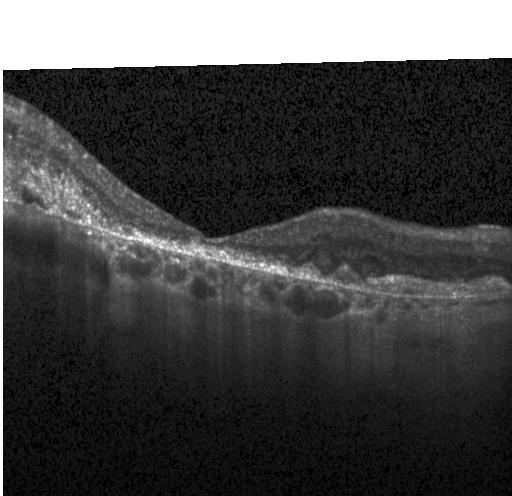
Fovea-centered. Spectral-domain optical coherence tomography. Optical coherence tomography B-scan.
This B-scan demonstrates choroidal neovascularization (CNV).